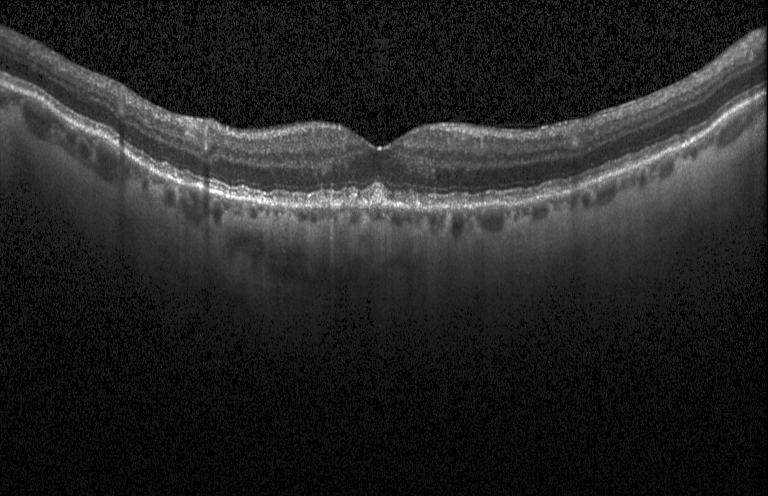

Spectral-domain OCT B-scan: multiple drusen.